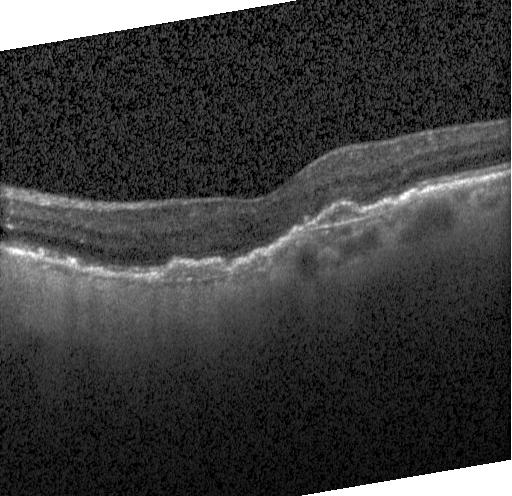
Retinal OCT cross-section showing choroidal neovascularization (CNV).